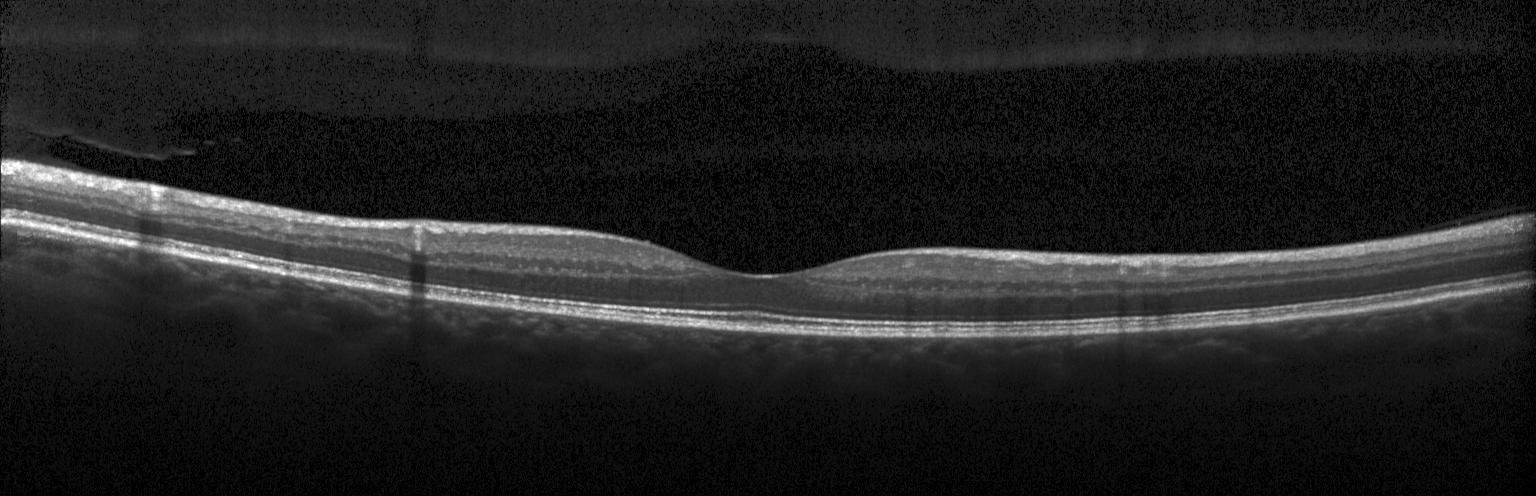 Instrument: Heidelberg Spectralis; centered on the fovea; retinal OCT B-scan — The scan shows no CNV, no DME, and no drusen.